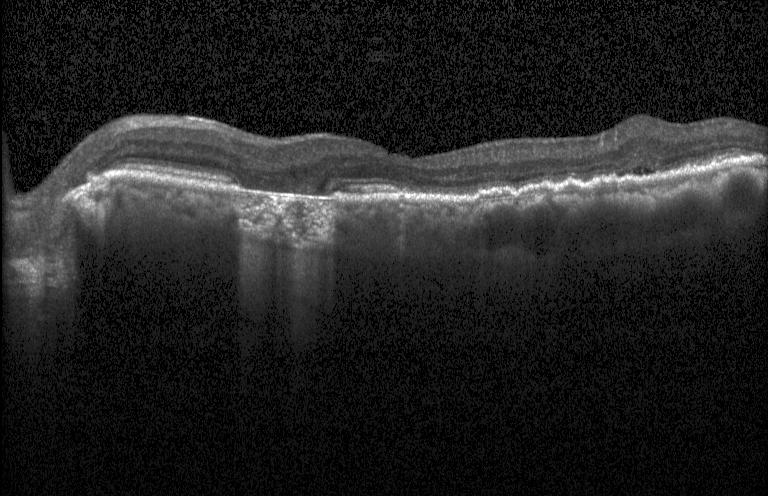
A choroidal neovascular membrane.